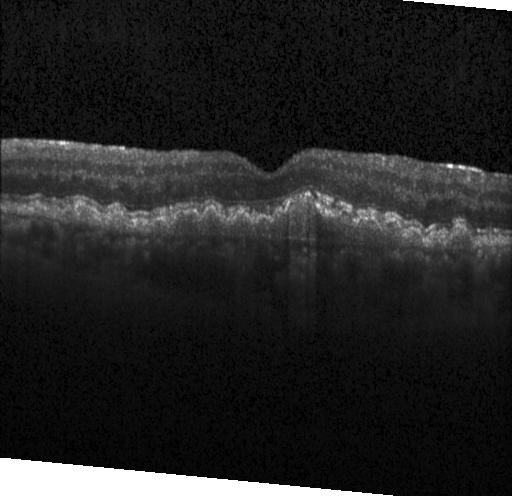
Fovea-centered · OCT B-scan
Diagnosis: a choroidal neovascular membrane.